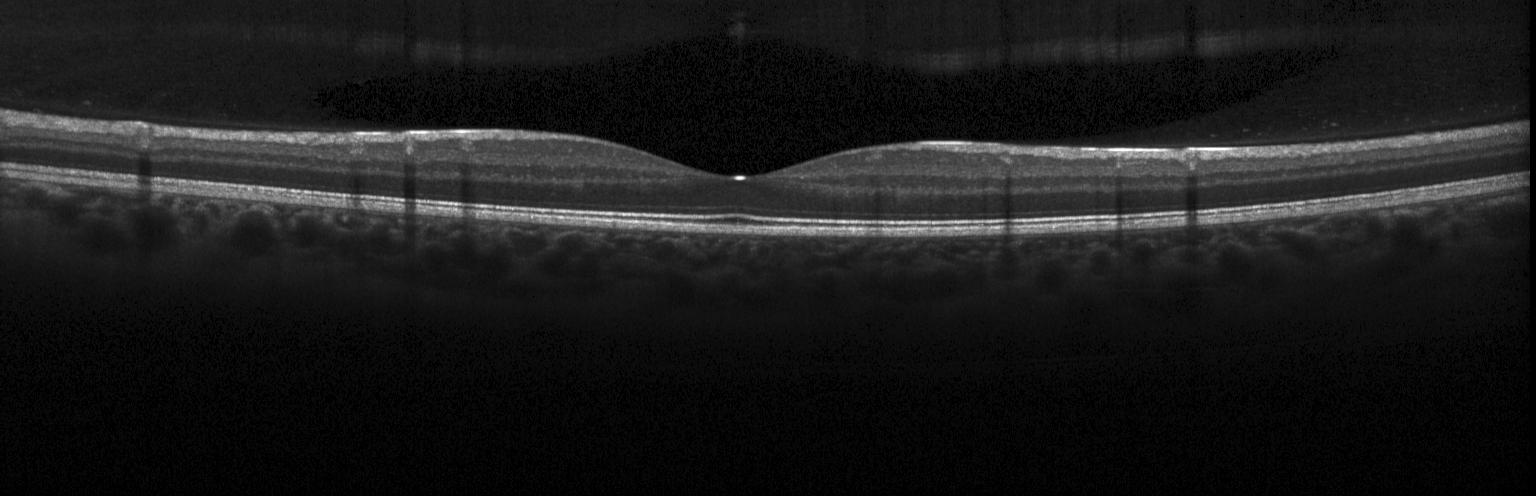 Spectral-domain OCT; OCT B-scan.
Neither CNV, DME, nor drusen.